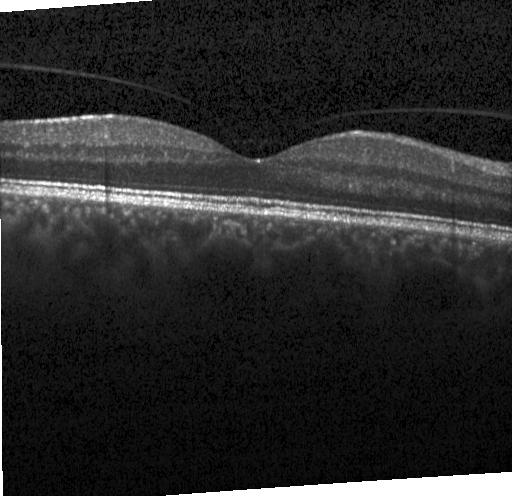

Impression: no CNV, DME, or drusen.